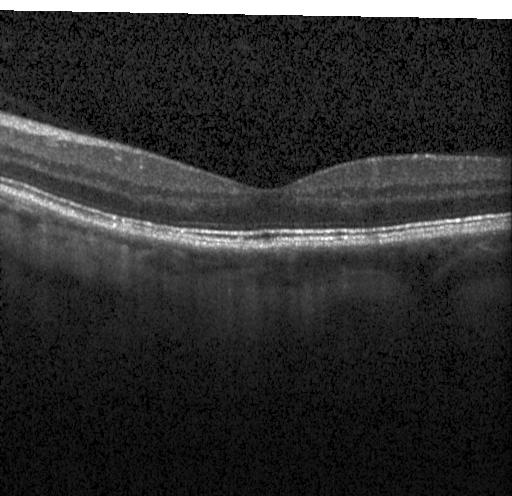

Retinal OCT cross-section. Macular scan. SD-OCT
Macular OCT: no choroidal neovascularization, diabetic macular edema, or drusen.